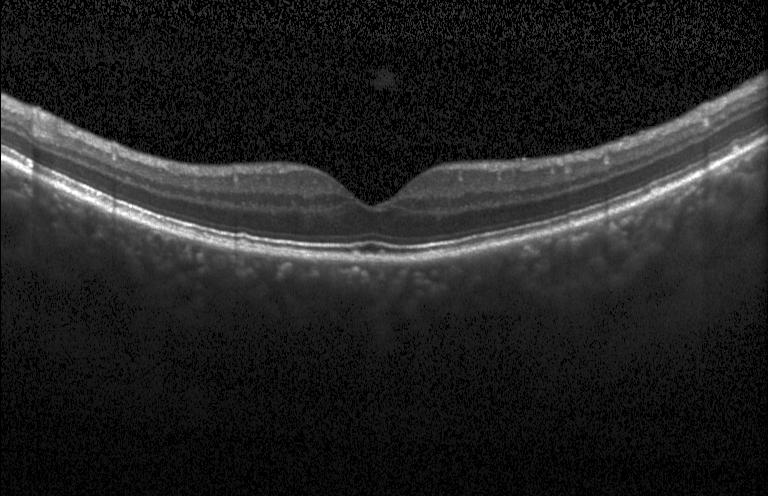 Macular scan; OCT line scan — Drusen.